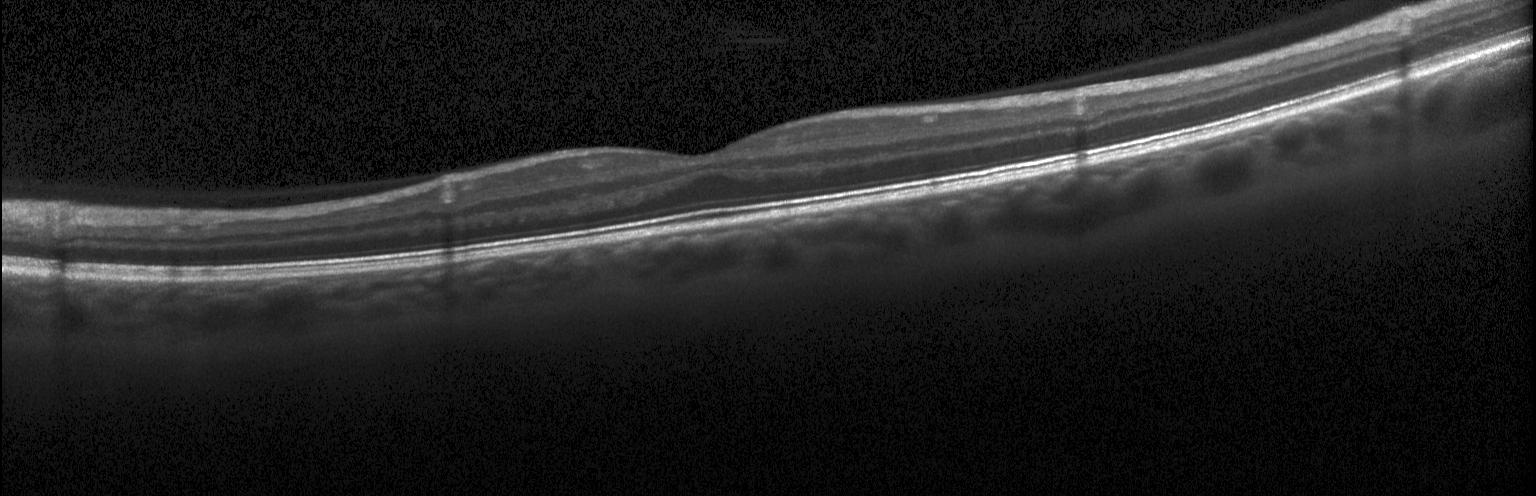
Horizontal scan through the fovea, spectral-domain optical coherence tomography, optical coherence tomography scan — Impression: neither choroidal neovascularization, diabetic macular edema, nor drusen.